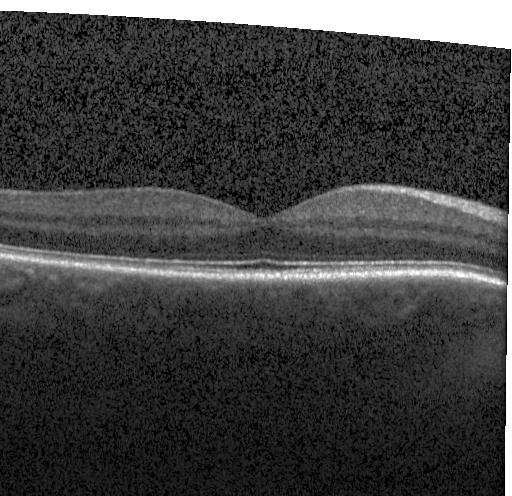 Centered on the fovea · OCT B-scan · spectral-domain OCT.
Finding: neither choroidal neovascularization, diabetic macular edema, nor drusen.